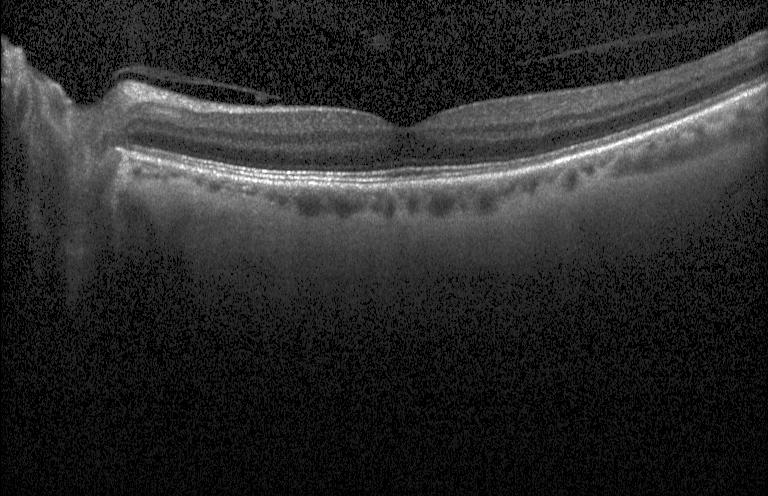

Impression: no choroidal neovascularization, no diabetic macular edema, and no drusen.